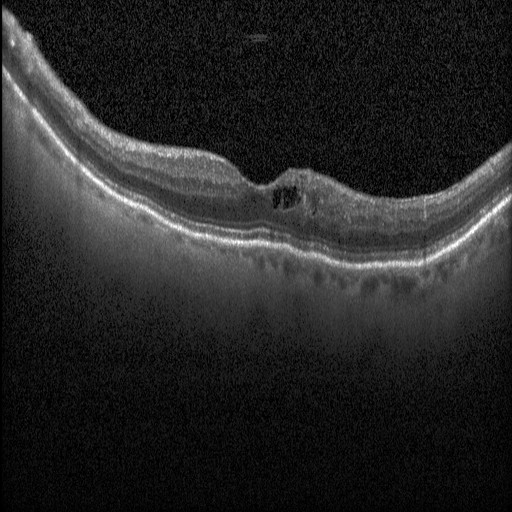 This B-scan demonstrates diabetic macular edema (DME).